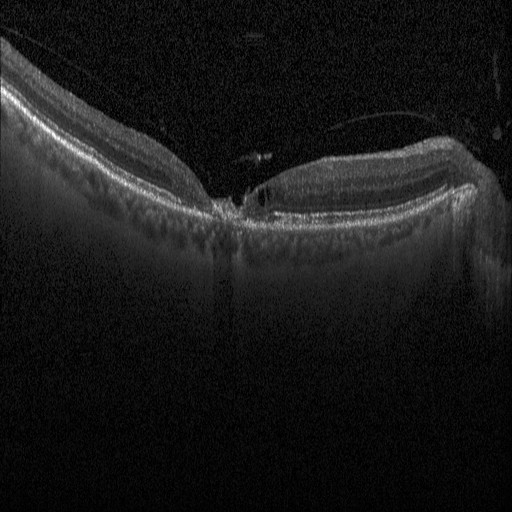
OCT B-scan; acquired on a Heidelberg Spectralis; spectral-domain OCT; horizontal scan through the fovea.
The scan shows diabetic macular edema.